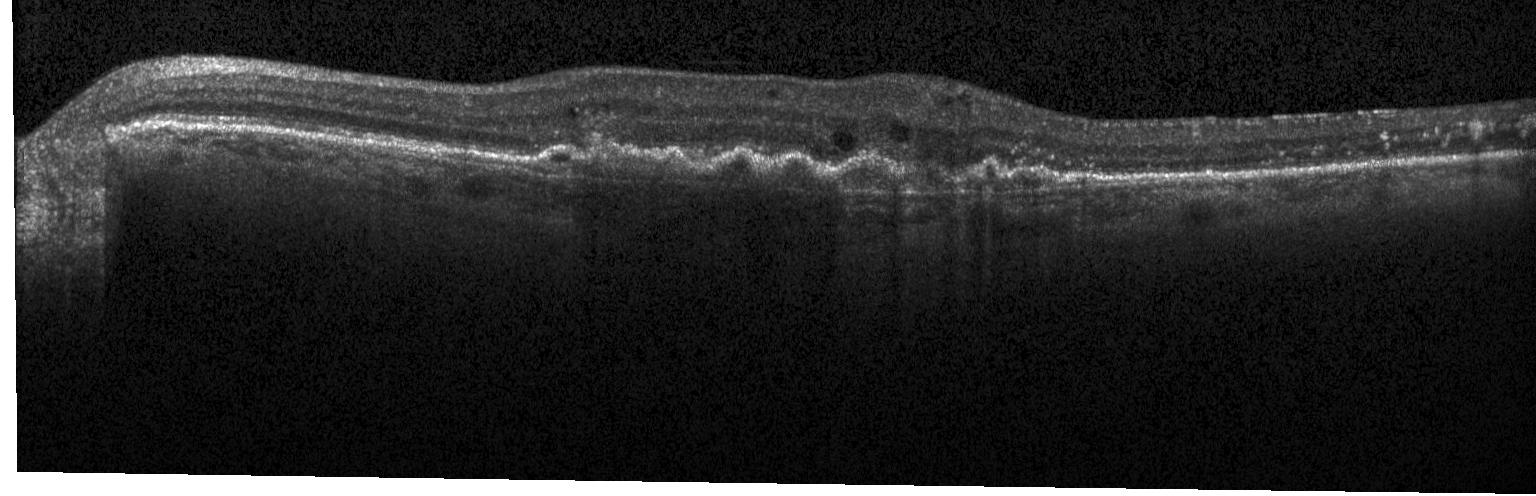
OCT finding: choroidal neovascularization (CNV).